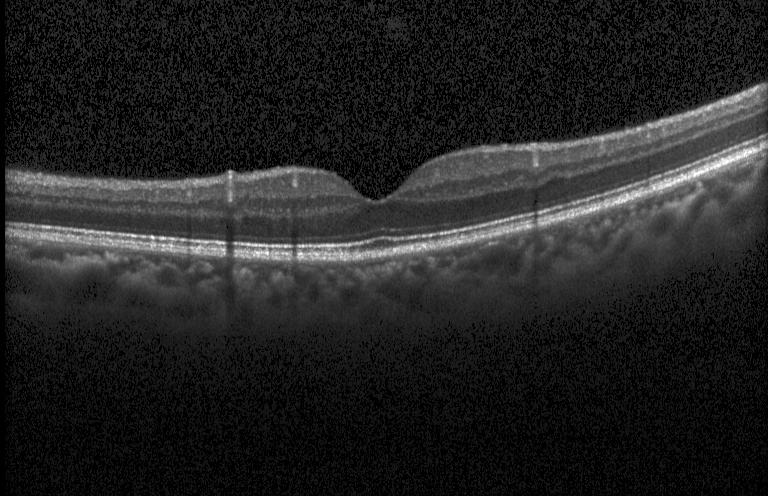
Acquired on a Heidelberg Spectralis, SD-OCT, through the macula, retinal OCT cross-section.
Diagnosis: neither choroidal neovascularization, diabetic macular edema, nor drusen.